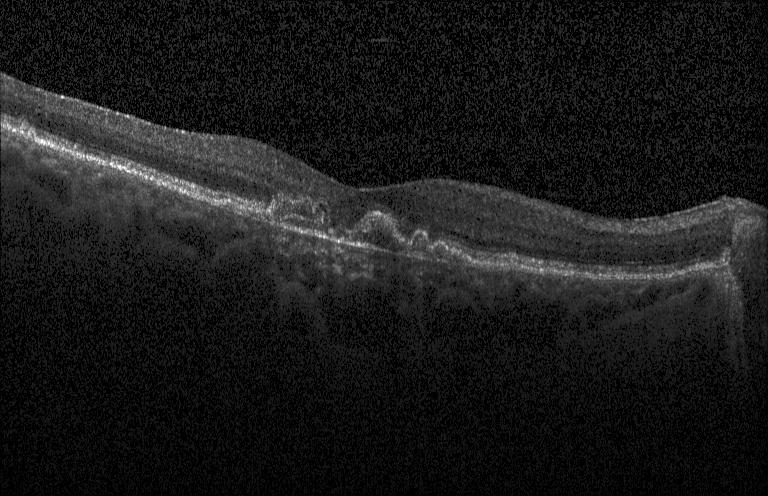

Spectral-domain OCT, acquired on a Heidelberg Spectralis, macular scan, retinal OCT B-scan. Choroidal neovascularization (CNV).